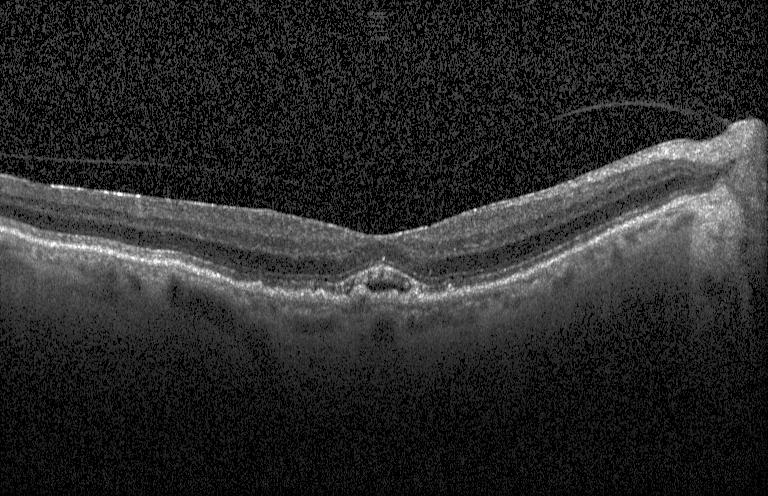

Diagnosis: a choroidal neovascular membrane.